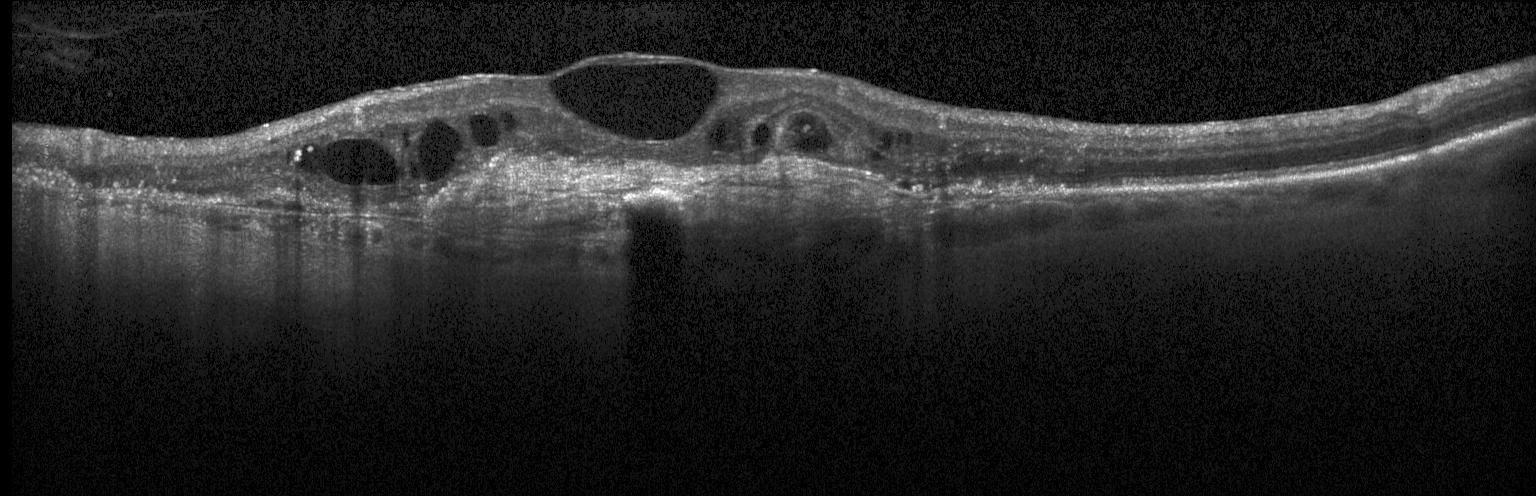 Impression: a choroidal neovascular membrane.